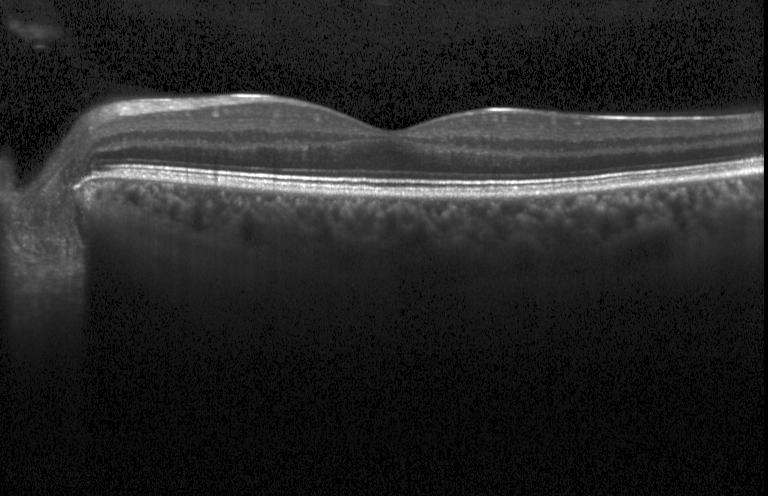
Macular OCT demonstrating neither CNV, DME, nor drusen.